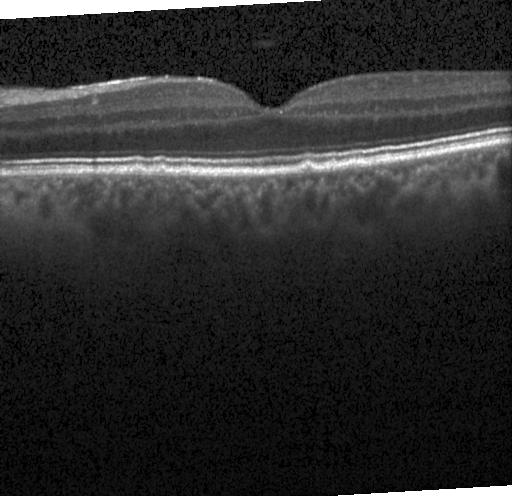
OCT finding: multiple drusen.